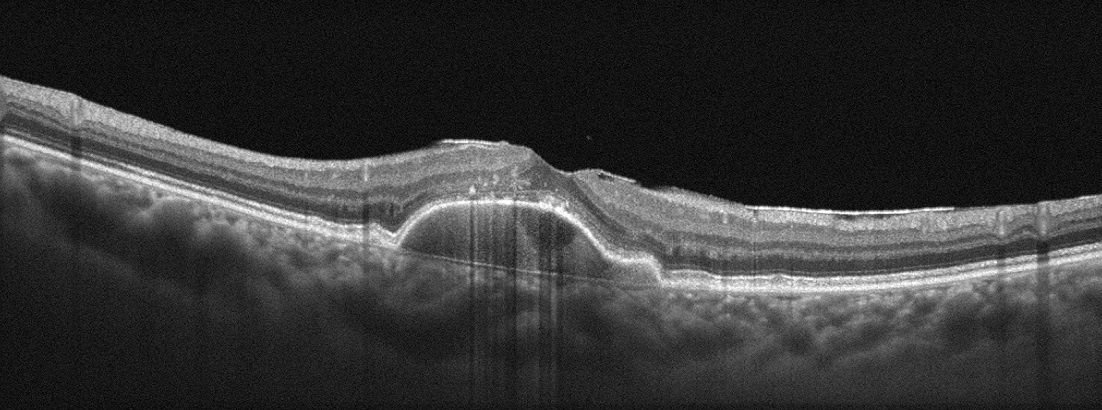
Finding: AMD.